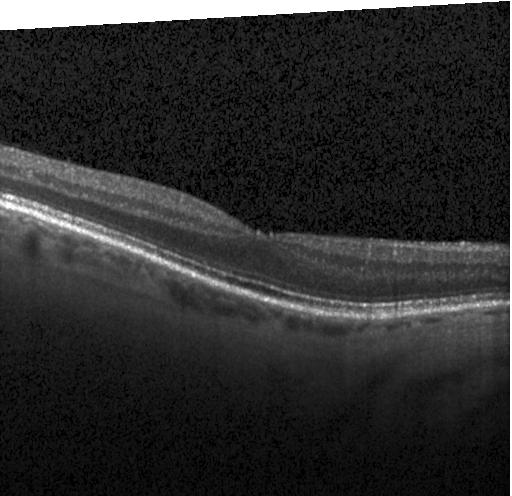
The scan shows no choroidal neovascularization, no diabetic macular edema, and no drusen.